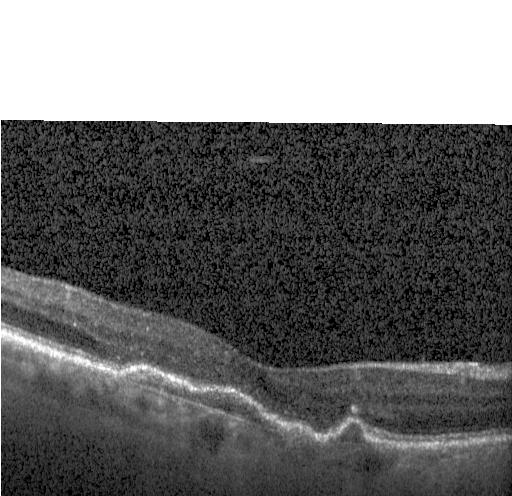
Assessment: choroidal neovascularization.